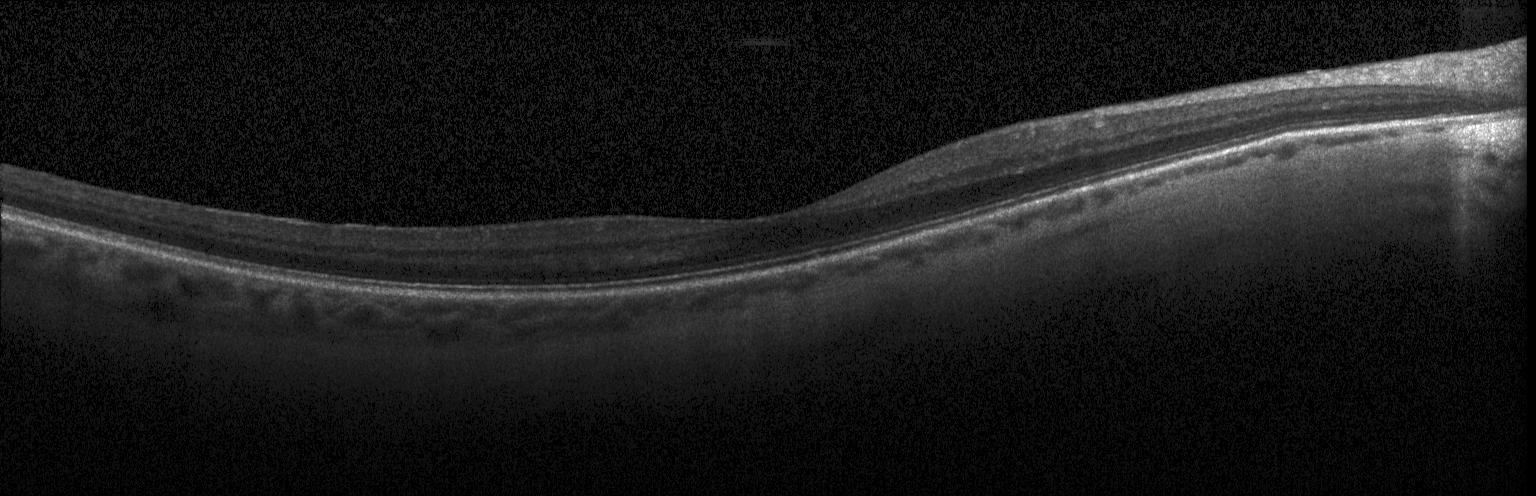

OCT line scan
This B-scan demonstrates neither choroidal neovascularization, diabetic macular edema, nor drusen.